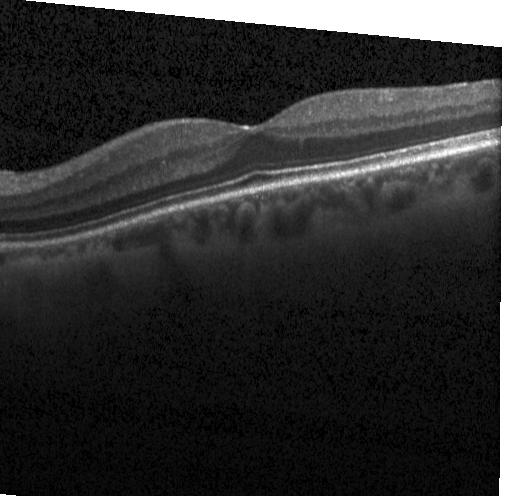
OCT B-scan · spectral-domain OCT
Macular OCT: no evidence of choroidal neovascularization, diabetic macular edema, or drusen.